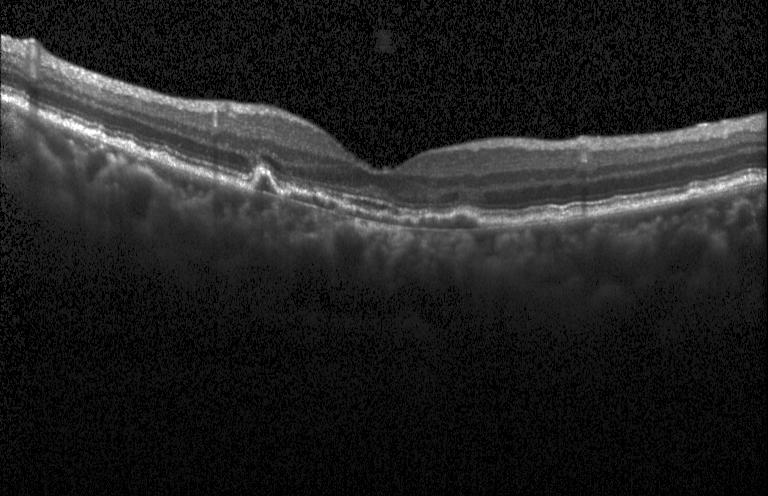
Dx: CNV.